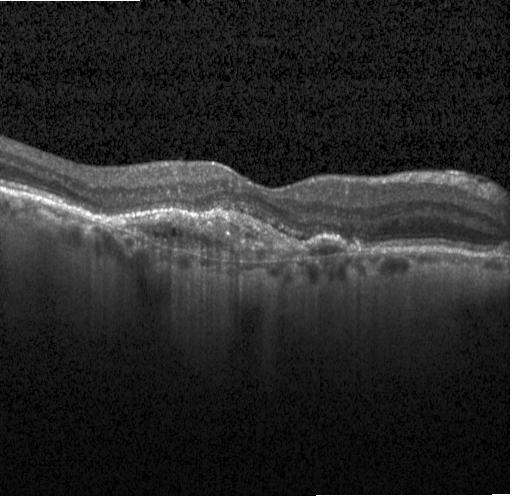
Impression: CNV.